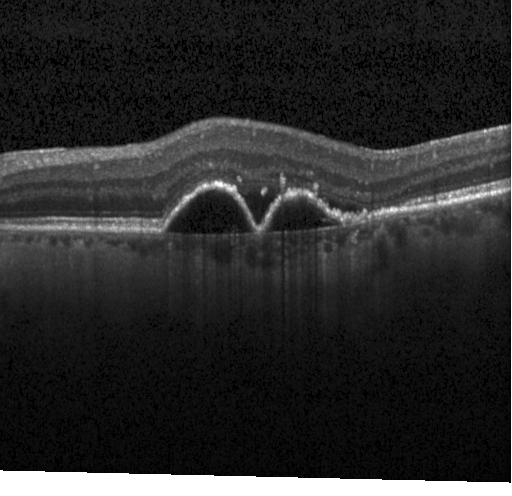 SD-OCT · OCT line scan · through the macula · instrument: Heidelberg Spectralis. Diagnosis: choroidal neovascularization.